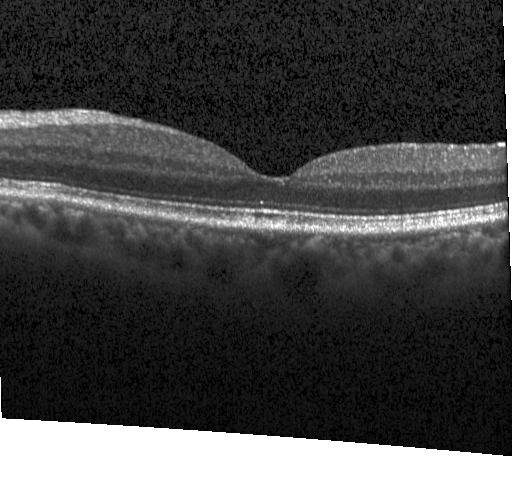
Diagnosis: no evidence of choroidal neovascularization, diabetic macular edema, or drusen.